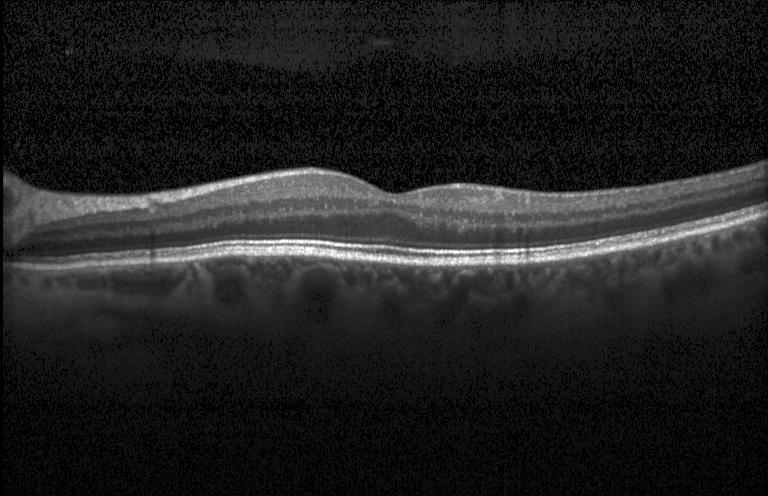

Heidelberg Spectralis · SD-OCT · optical coherence tomography B-scan.
The scan shows no choroidal neovascularization, diabetic macular edema, or drusen.